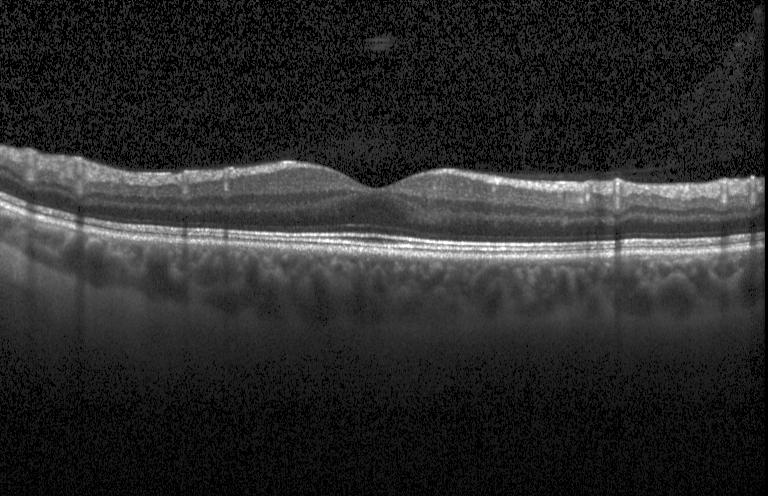

OCT finding: no choroidal neovascularization, diabetic macular edema, or drusen.